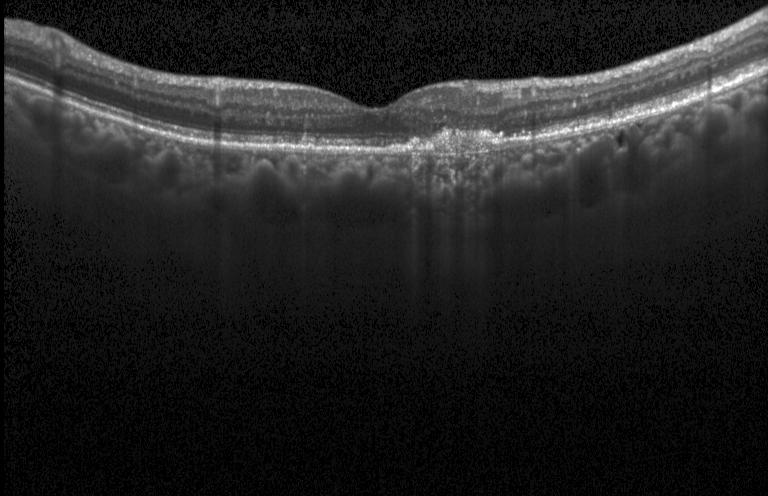 Optical coherence tomography B-scan. Heidelberg Spectralis. Centered on the fovea. Spectral-domain optical coherence tomography.
Choroidal neovascularization.